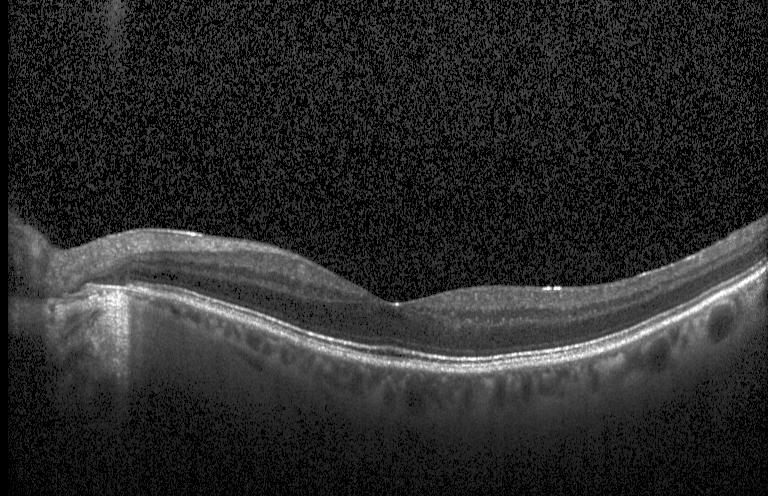 Spectral-domain optical coherence tomography, horizontal scan through the fovea, optical coherence tomography B-scan, Heidelberg Spectralis OCT system. OCT finding: no evidence of CNV, DME, or drusen.